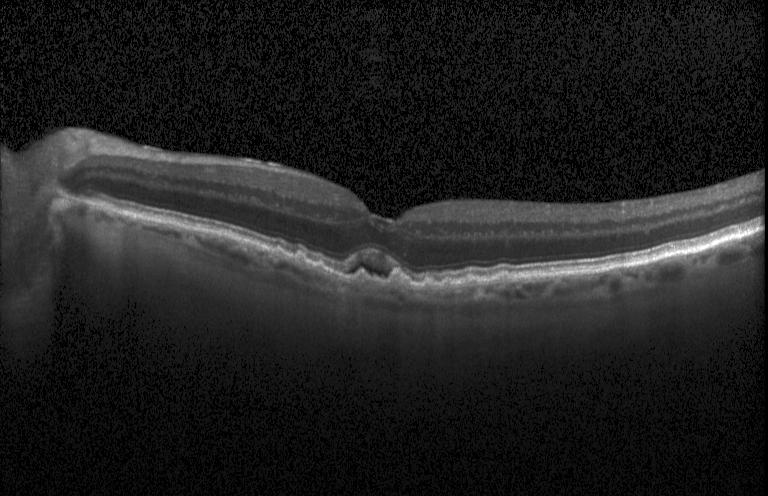

OCT B-scan. Finding: choroidal neovascularization.